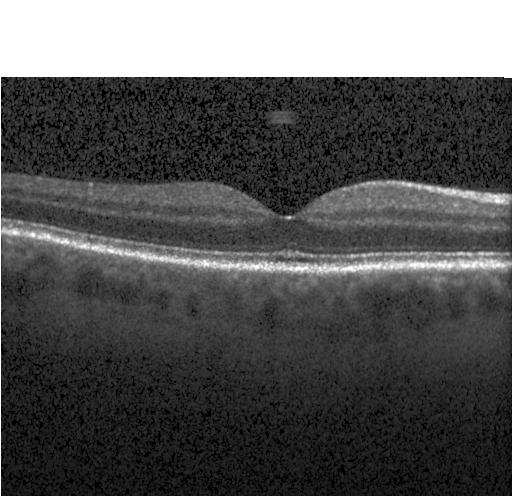
Impression: no evidence of choroidal neovascularization, diabetic macular edema, or drusen.